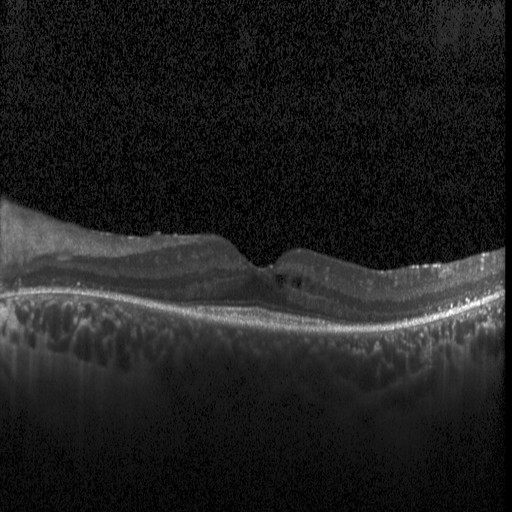

OCT line scan; SD-OCT
OCT finding: diabetic macular edema.